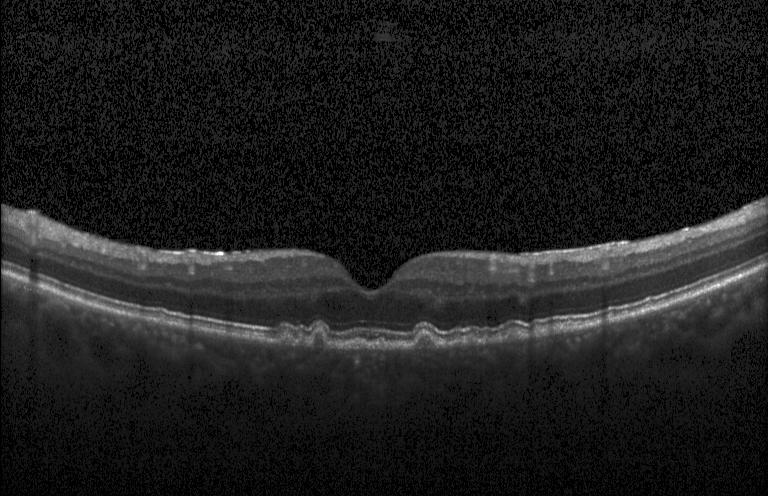 Dx: sub-RPE drusenoid deposits.